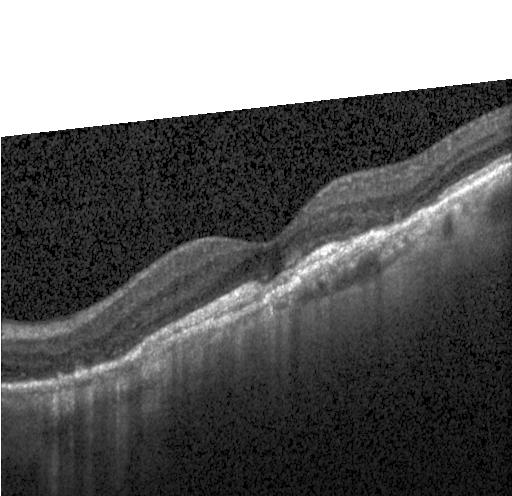

Optical coherence tomography scan
Impression: a choroidal neovascular membrane.